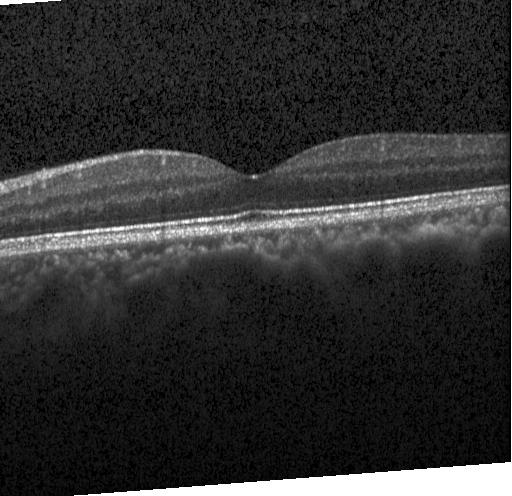
Macular OCT demonstrating neither CNV, DME, nor drusen.